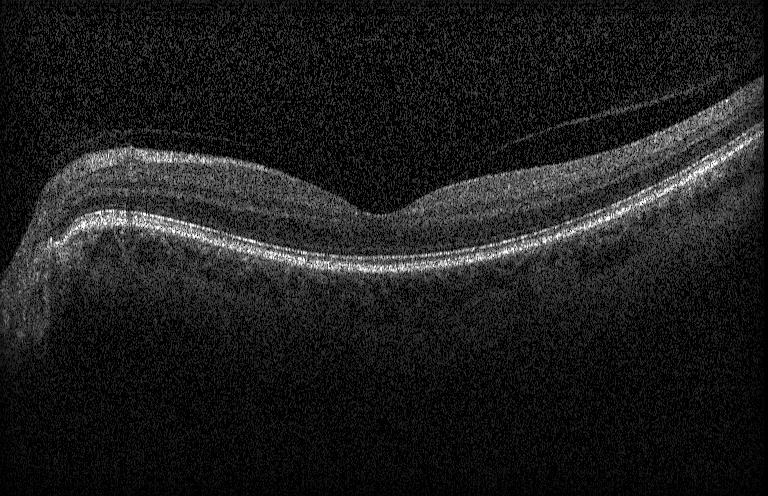 Macular scan, optical coherence tomography B-scan.
Diagnosis: no choroidal neovascularization, no diabetic macular edema, and no drusen.